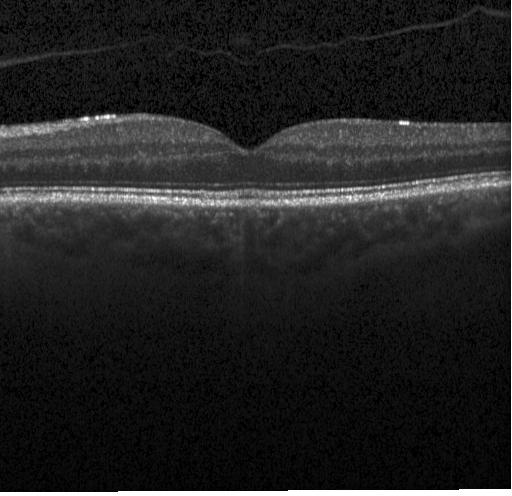
Dx: neither choroidal neovascularization, diabetic macular edema, nor drusen.